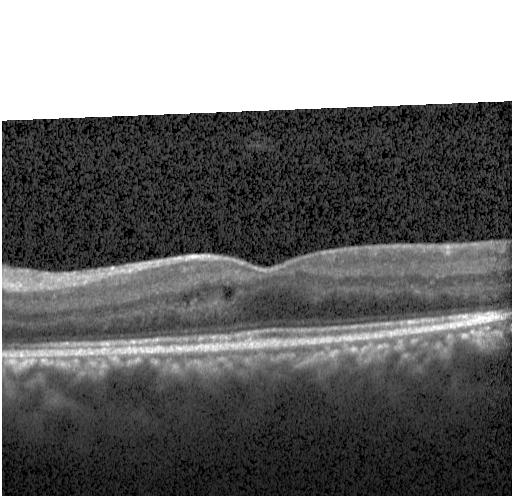 Retinal OCT cross-section showing diabetic macular edema (DME).